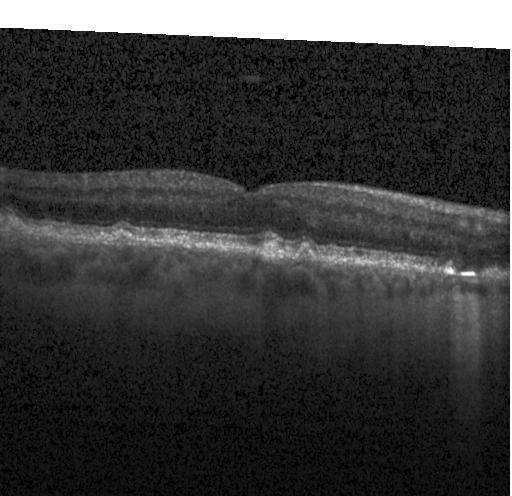 Macular scan; retinal OCT cross-section; spectral-domain optical coherence tomography; Heidelberg Spectralis OCT system — Assessment: drusen.